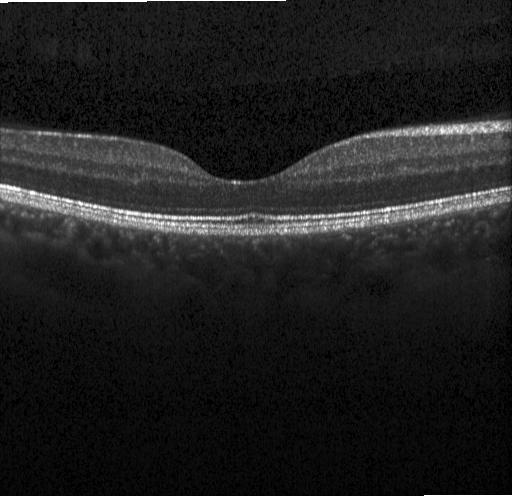

Heidelberg Spectralis OCT system. Spectral-domain OCT. OCT B-scan. Horizontal scan through the fovea.
Diagnosis: no evidence of choroidal neovascularization, diabetic macular edema, or drusen.